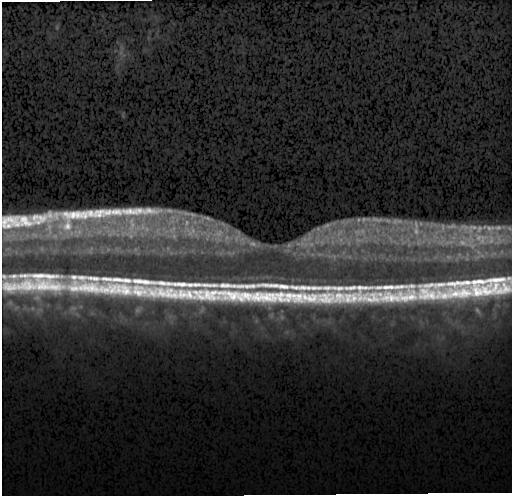

OCT B-scan; spectral-domain optical coherence tomography; fovea-centered. Finding: no CNV, no DME, and no drusen.